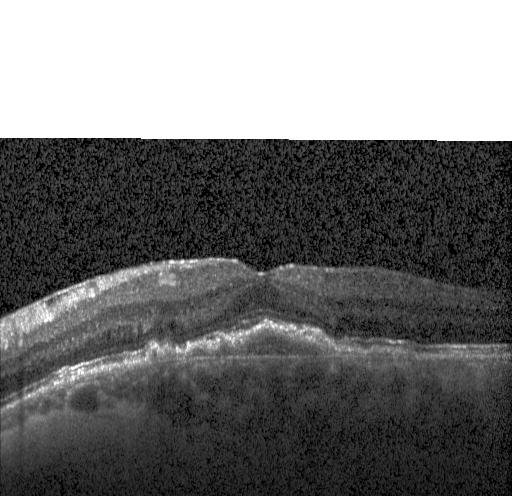 Diagnosis: a choroidal neovascular membrane.